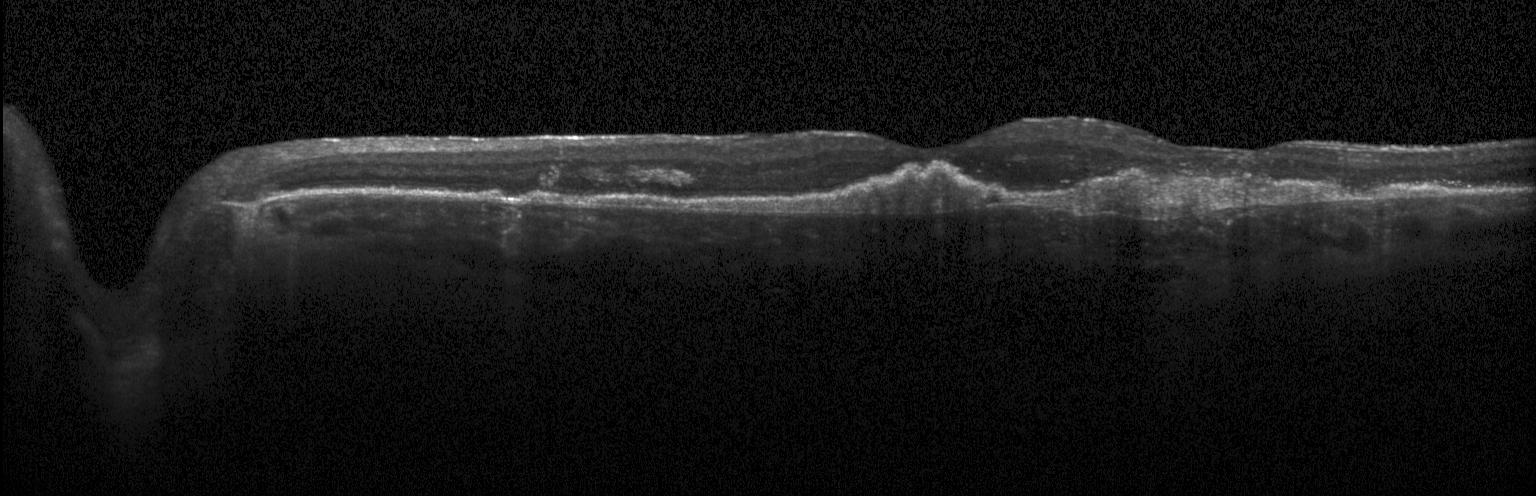

Optical coherence tomography B-scan
Finding: a choroidal neovascular membrane.